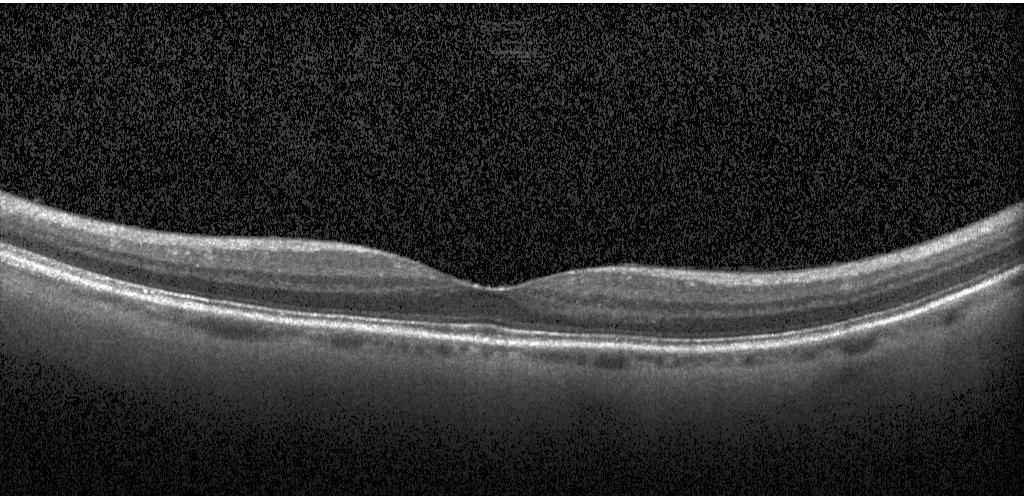 Impression: no choroidal neovascularization, diabetic macular edema, or drusen.